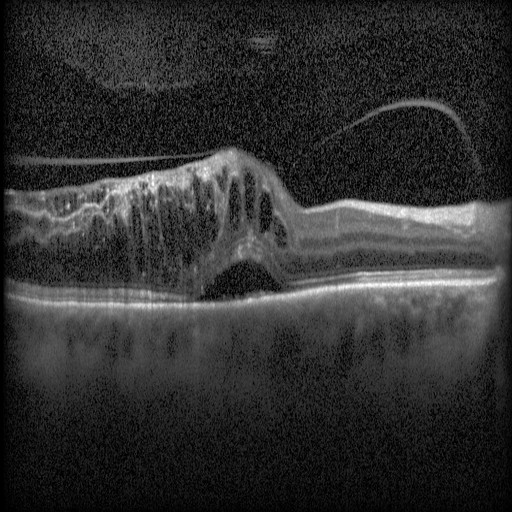 Impression: DME.